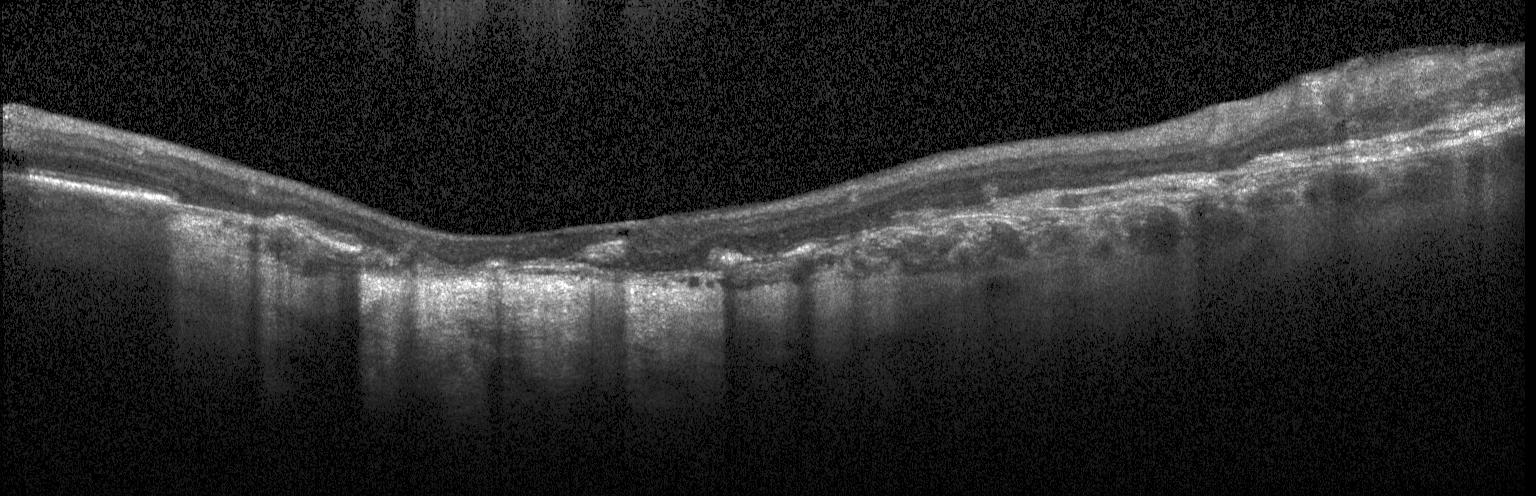
Diagnosis: a choroidal neovascular membrane.